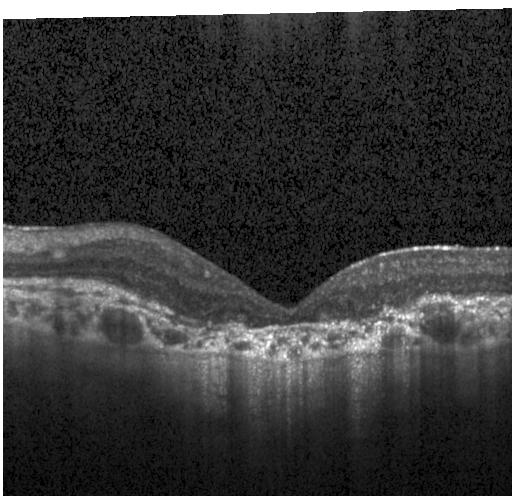

Dx: choroidal neovascularization (CNV).